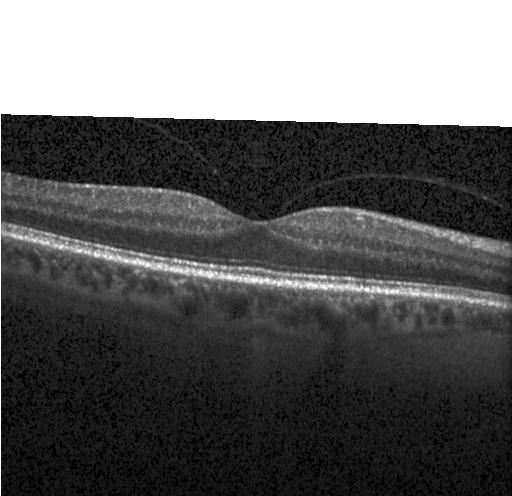
Retinal OCT cross-section, instrument: Heidelberg Spectralis, spectral-domain OCT.
No evidence of choroidal neovascularization, diabetic macular edema, or drusen.